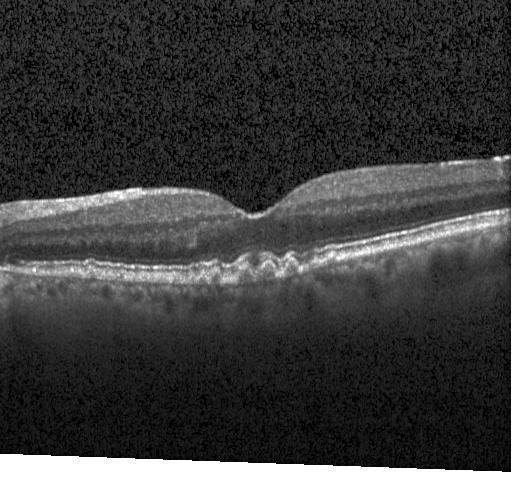
Finding: drusen.